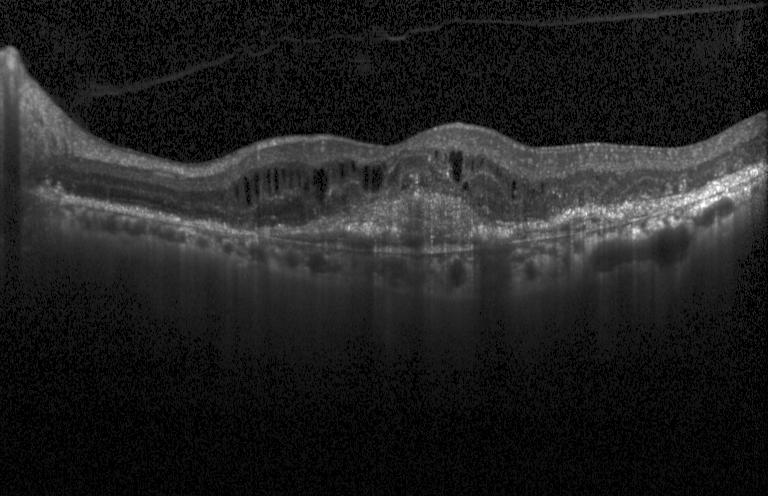 OCT line scan — This B-scan demonstrates a choroidal neovascular membrane.